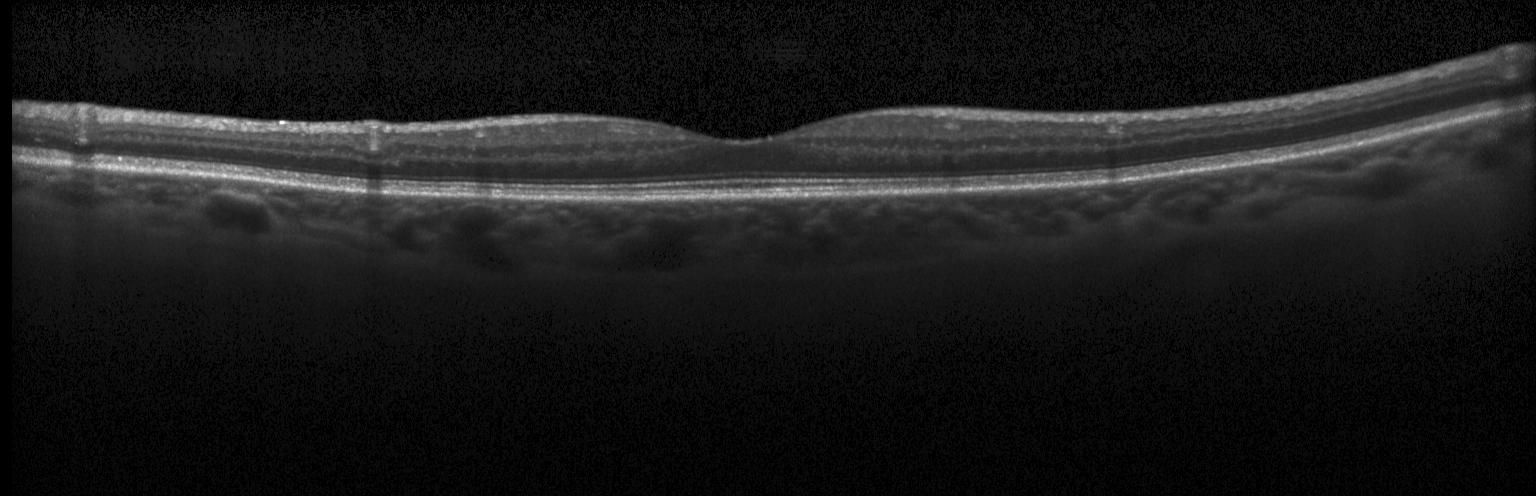 Spectral-domain optical coherence tomography. Fovea-centered. Optical coherence tomography B-scan
Dx: no evidence of choroidal neovascularization, diabetic macular edema, or drusen.